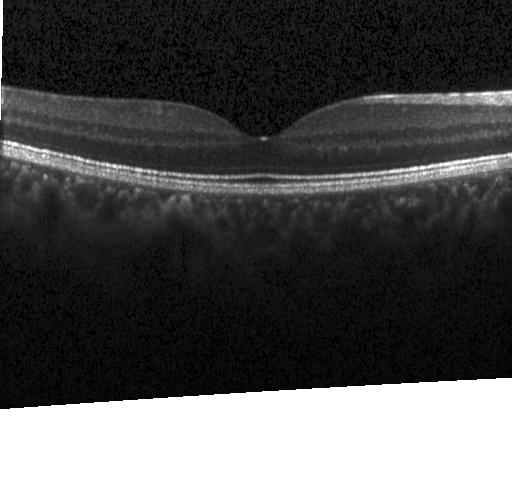 Impression: neither choroidal neovascularization, diabetic macular edema, nor drusen.